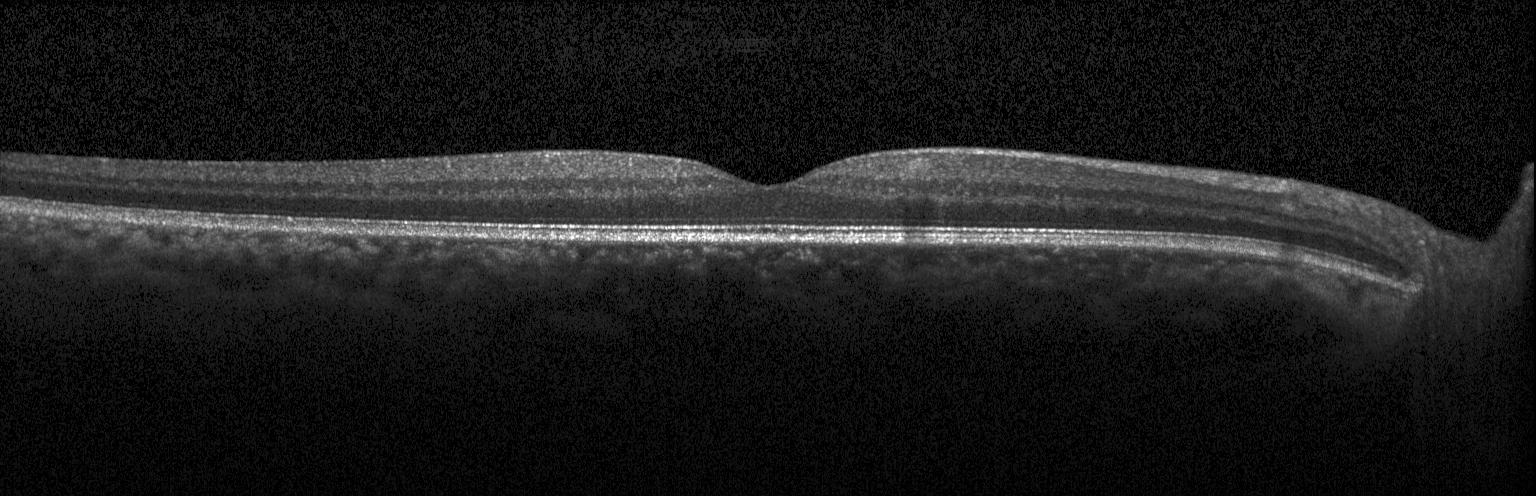

Retinal OCT cross-section · spectral-domain optical coherence tomography. Dx: no choroidal neovascularization, no diabetic macular edema, and no drusen.